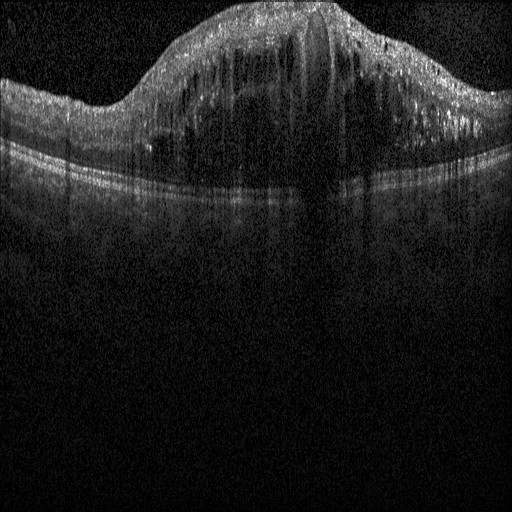 Retinal OCT cross-section showing diabetic macular edema.